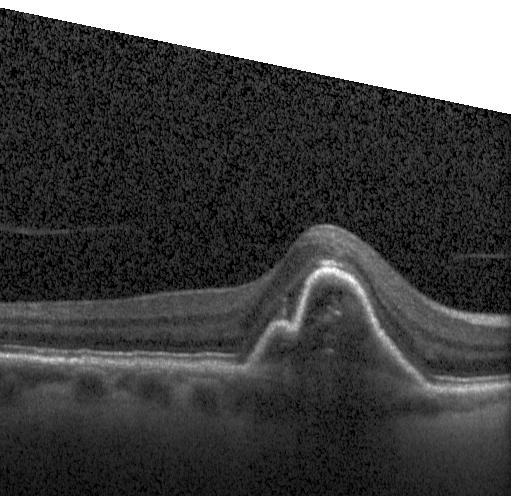

Macular OCT demonstrating a choroidal neovascular membrane.